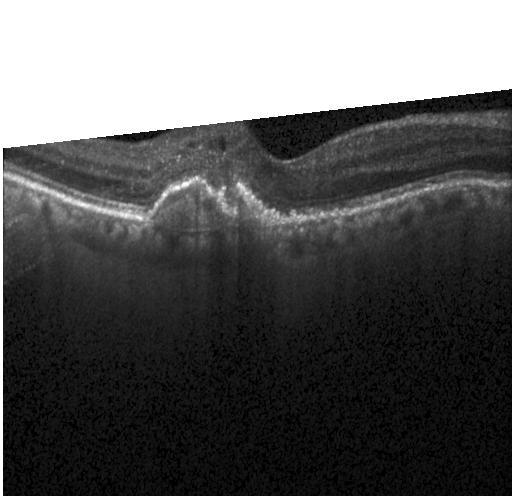 Impression: a choroidal neovascular membrane.